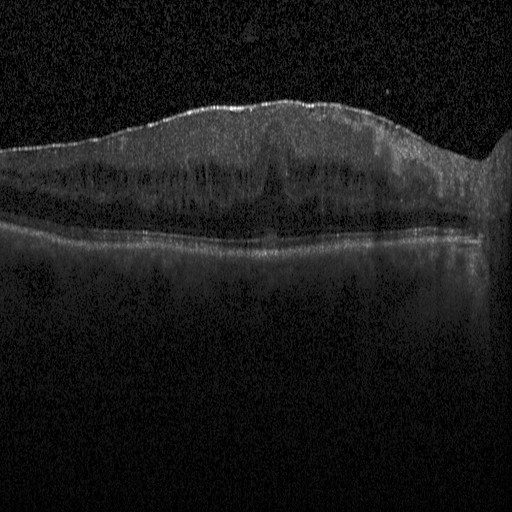

Optical coherence tomography scan
Finding: diabetic macular edema (DME).